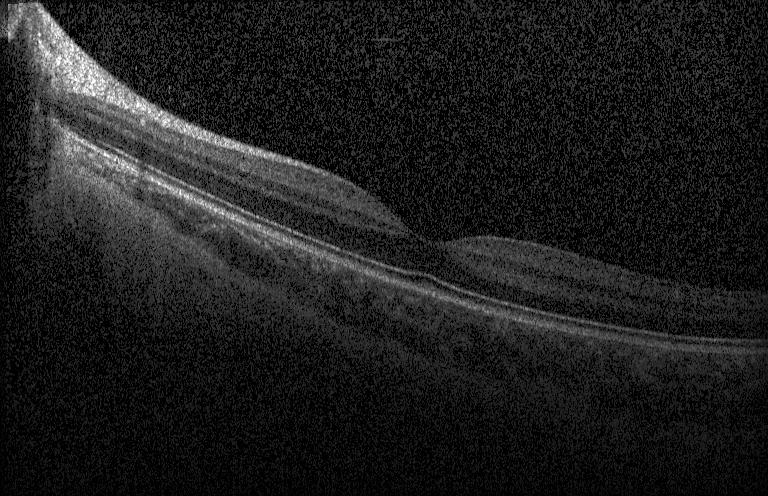
No evidence of choroidal neovascularization, diabetic macular edema, or drusen.